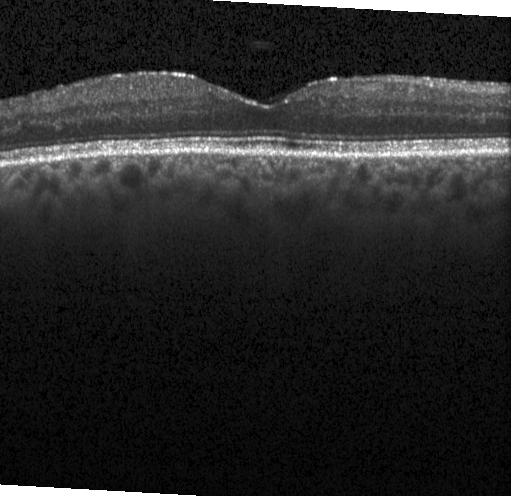
Retinal OCT cross-section showing no choroidal neovascularization, diabetic macular edema, or drusen.